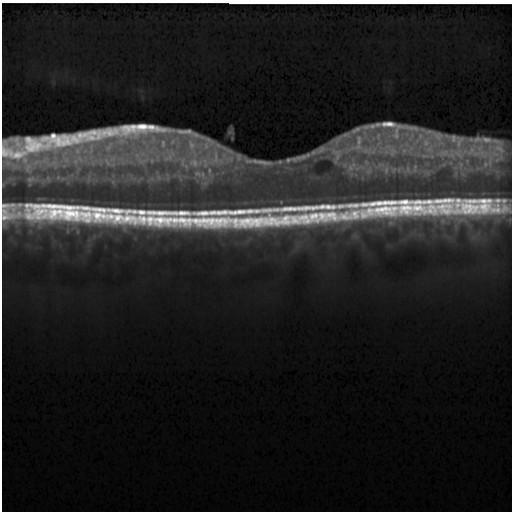

Optical coherence tomography scan; spectral-domain optical coherence tomography; fovea-centered; instrument: Heidelberg Spectralis. Diagnosis: DME.